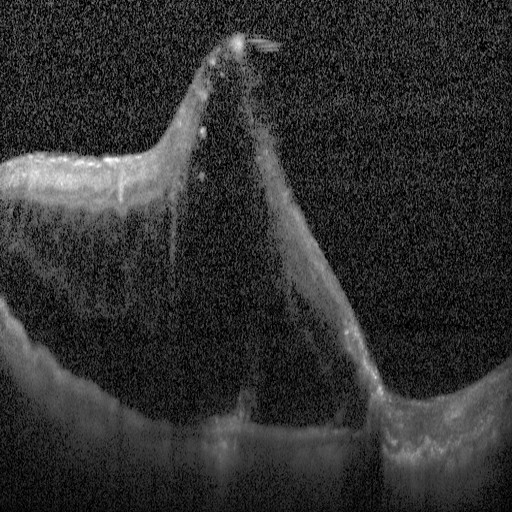
Heidelberg Spectralis, horizontal scan through the fovea, spectral-domain optical coherence tomography, optical coherence tomography B-scan
Diagnosis: diabetic macular edema (DME).